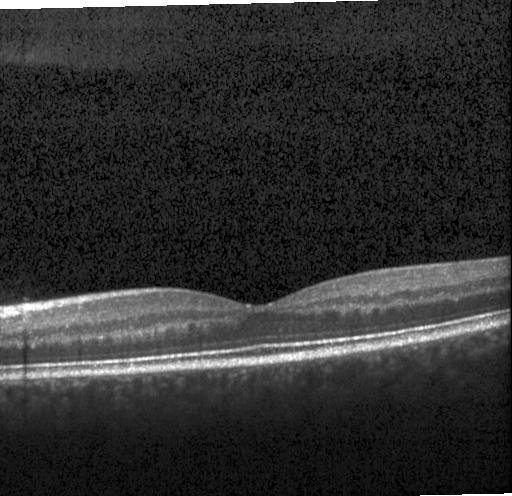 Optical coherence tomography B-scan
Macular OCT: no choroidal neovascularization, no diabetic macular edema, and no drusen.